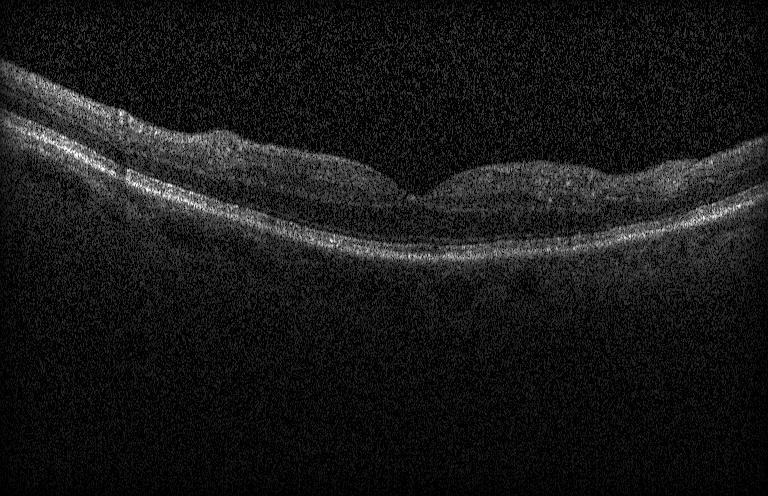

Optical coherence tomography scan · acquired on a Heidelberg Spectralis. Dx: neither CNV, DME, nor drusen.